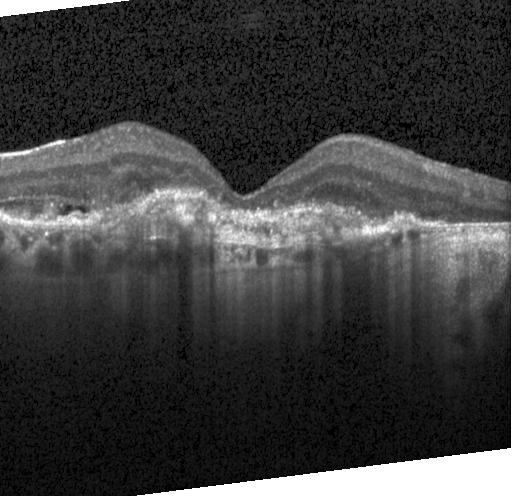

OCT line scan
Impression: choroidal neovascularization.